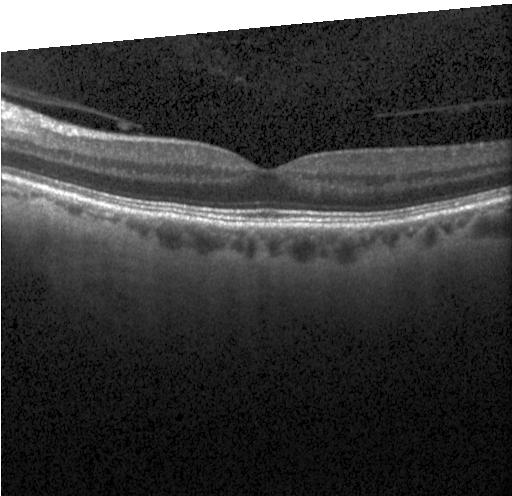

Retinal OCT B-scan. Spectral-domain optical coherence tomography — This B-scan demonstrates no choroidal neovascularization, diabetic macular edema, or drusen.